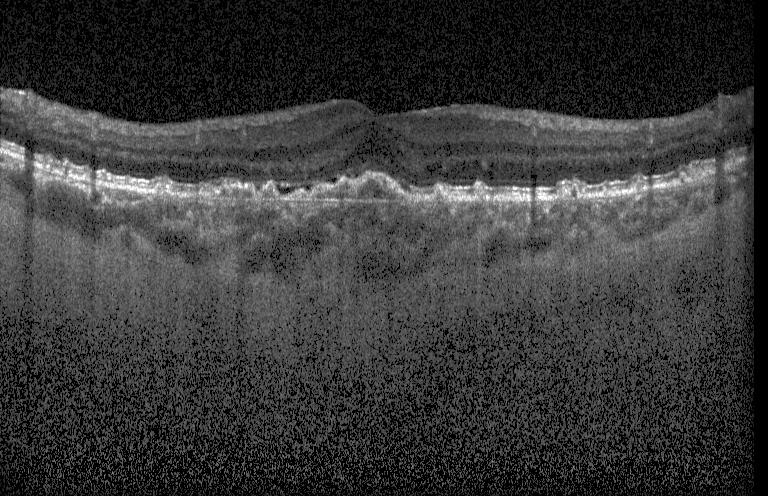 OCT line scan. Diagnosis: CNV.